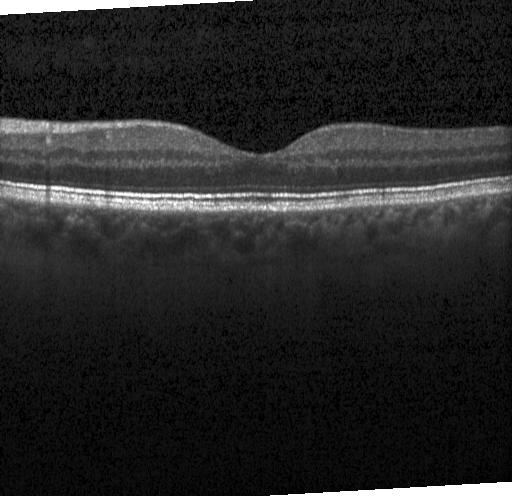

Acquired on a Heidelberg Spectralis; spectral-domain OCT; optical coherence tomography B-scan; centered on the fovea — Macular OCT: neither choroidal neovascularization, diabetic macular edema, nor drusen.